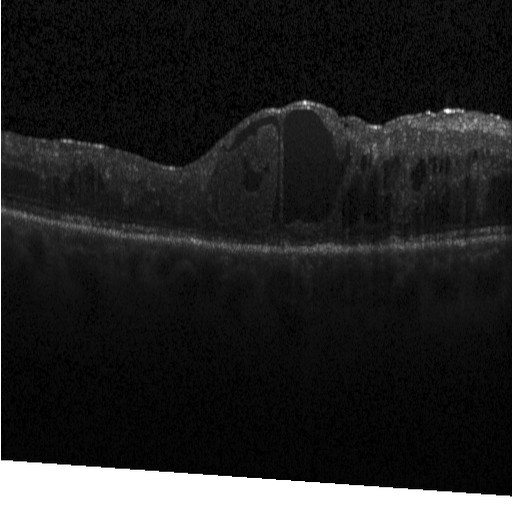

Fovea-centered · spectral-domain optical coherence tomography · retinal OCT B-scan · acquired on a Heidelberg Spectralis — Impression: diabetic macular edema.